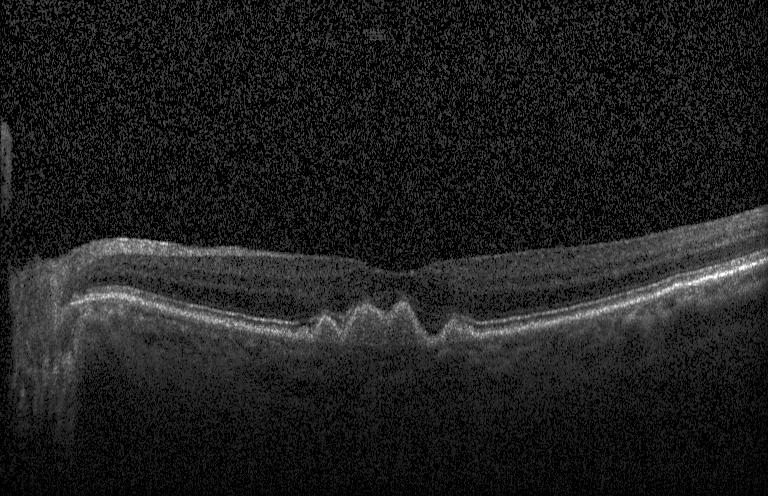 Diagnosis: multiple drusen.